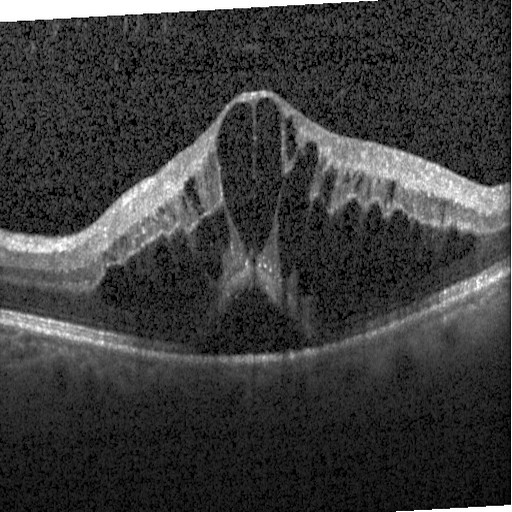
Assessment: DME.